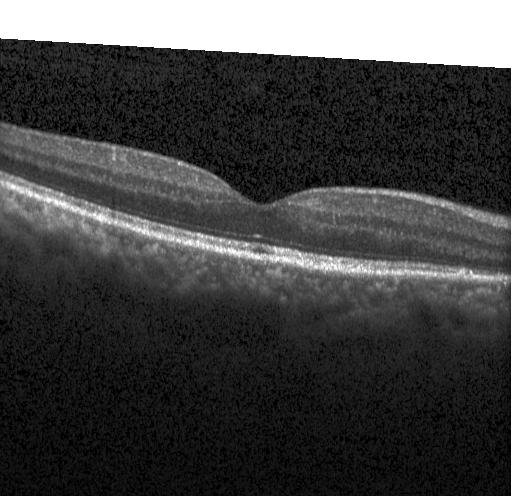
Finding: no CNV, no DME, and no drusen.